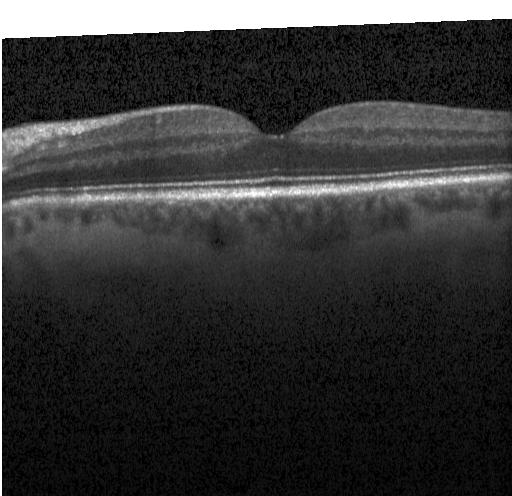

Finding: no CNV, no DME, and no drusen.